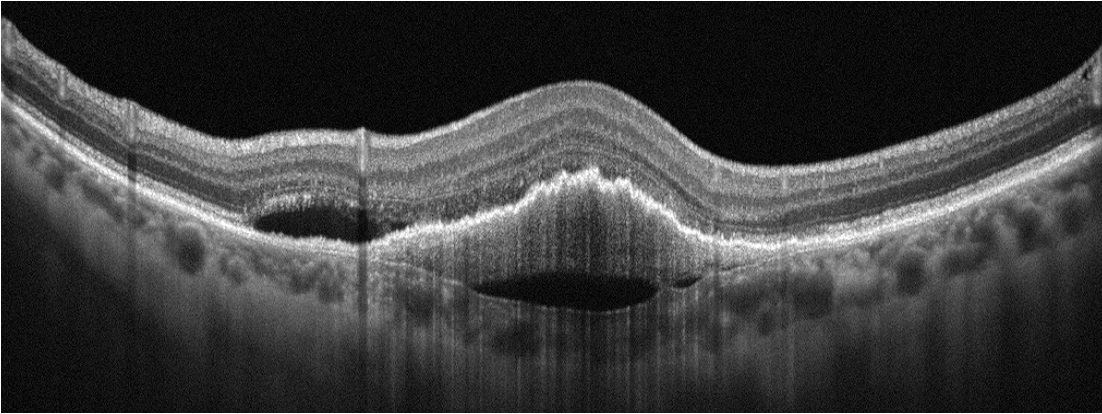 Acquired on an Optovue Avanti RTVue XR; OCT B-scan; through the macula
OCT finding: AMD.